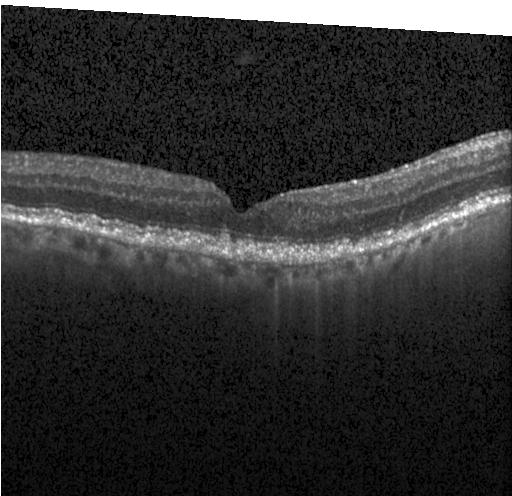
Drusen.